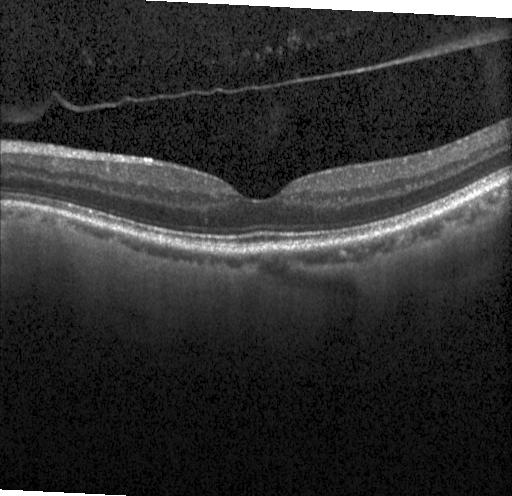 Centered on the fovea, Heidelberg Spectralis OCT system, OCT line scan, SD-OCT. Neither CNV, DME, nor drusen.